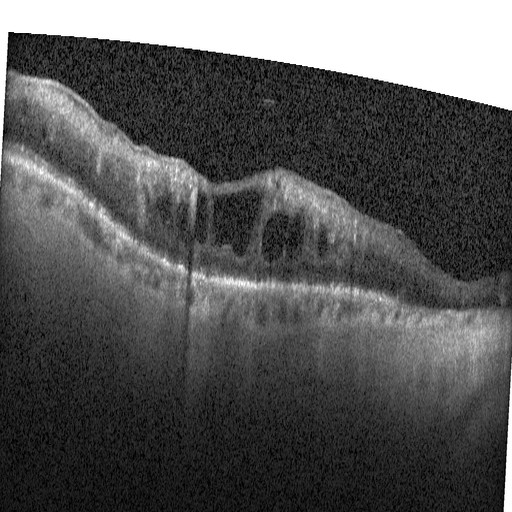

Retinal OCT cross-section showing diabetic macular edema.